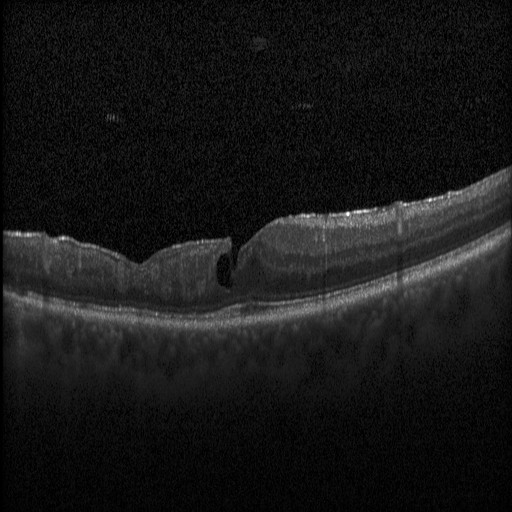 Horizontal scan through the fovea · acquired on a Heidelberg Spectralis · retinal OCT cross-section · spectral-domain optical coherence tomography — Finding: diabetic macular edema.